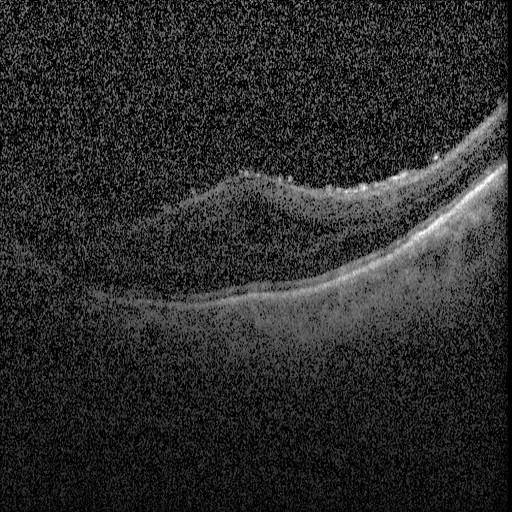
Macular scan; optical coherence tomography scan
Finding: diabetic macular edema.